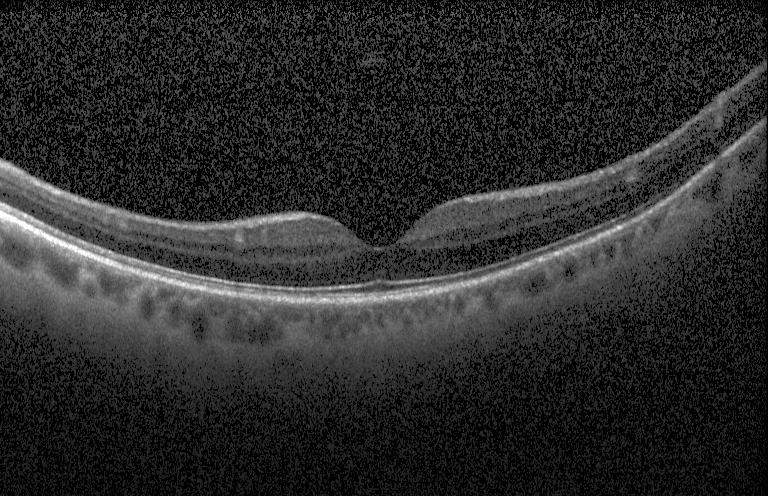

OCT line scan.
The scan shows no choroidal neovascularization, diabetic macular edema, or drusen.